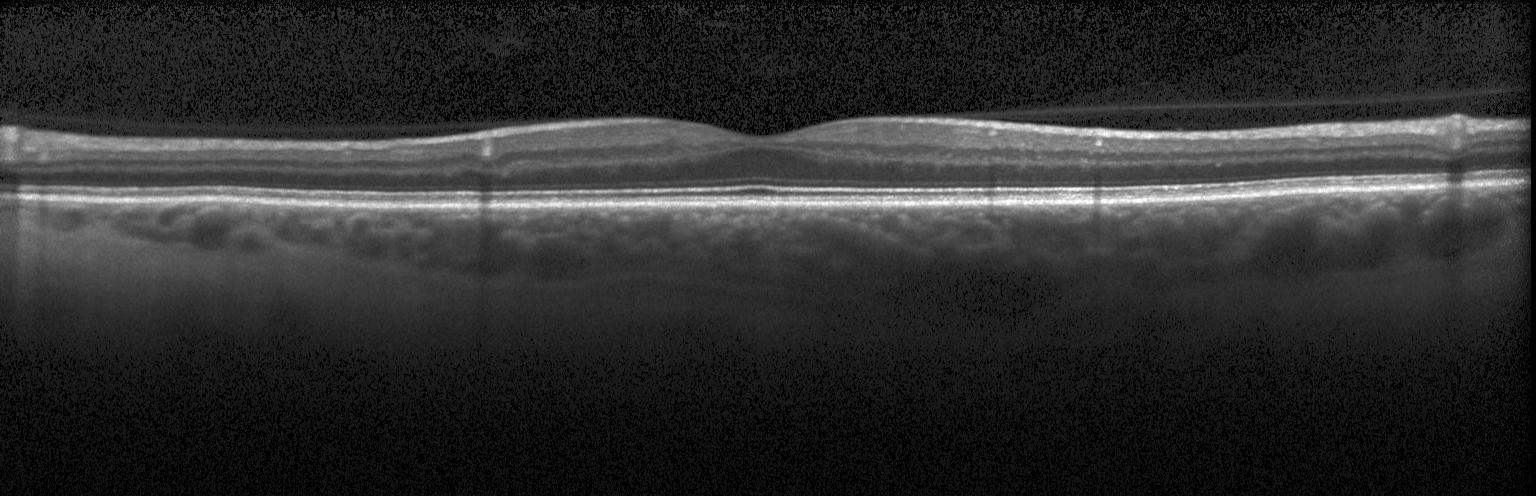

Macular OCT demonstrating no evidence of CNV, DME, or drusen.